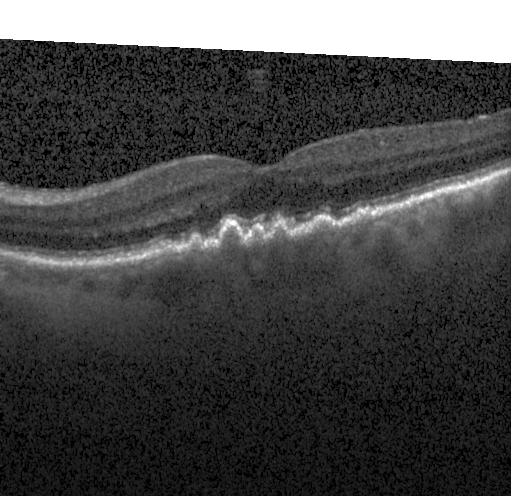 Horizontal scan through the fovea; acquired on a Heidelberg Spectralis; retinal OCT cross-section
Diagnosis: sub-RPE drusenoid deposits.